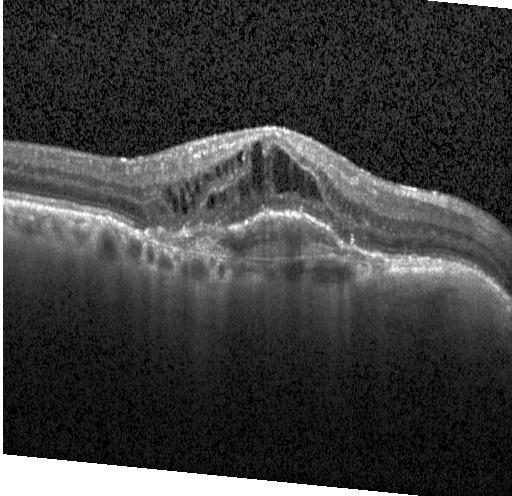 Retinal OCT cross-section
Impression: choroidal neovascularization.